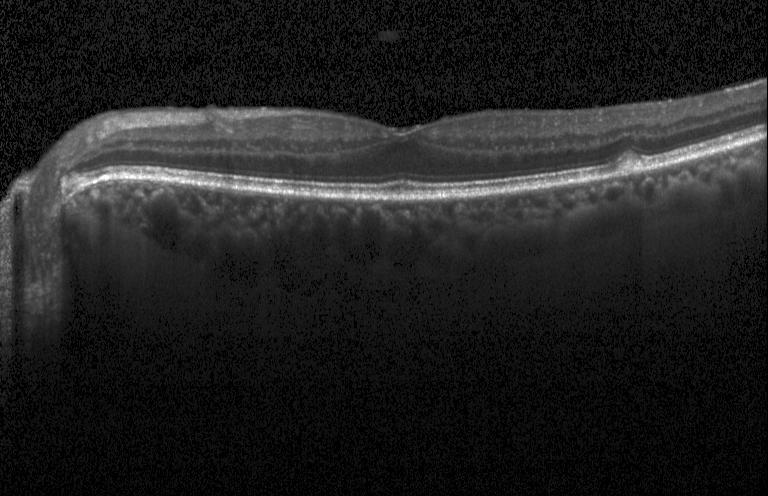

Finding: drusen.